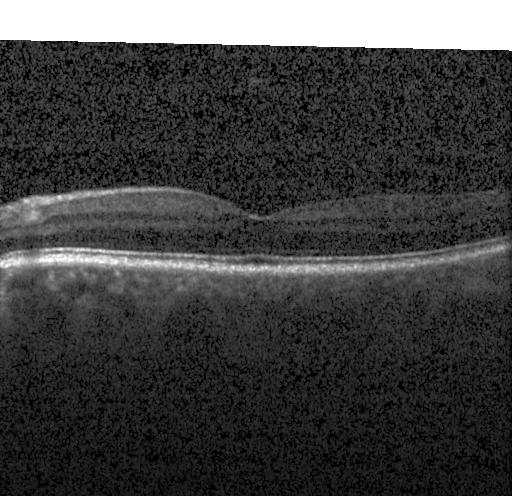
OCT B-scan showing neither choroidal neovascularization, diabetic macular edema, nor drusen.